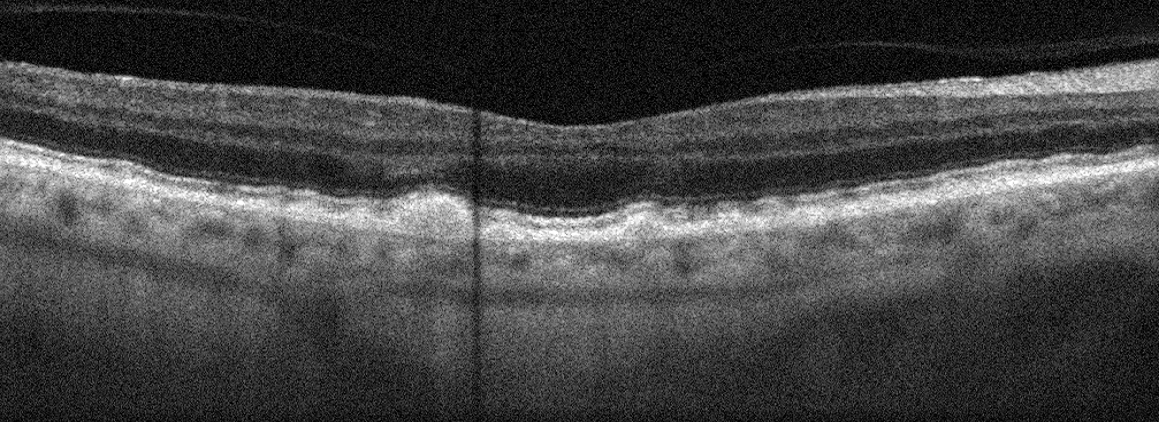

Optical coherence tomography B-scan · oculus dexter
Diagnosis: AMD.